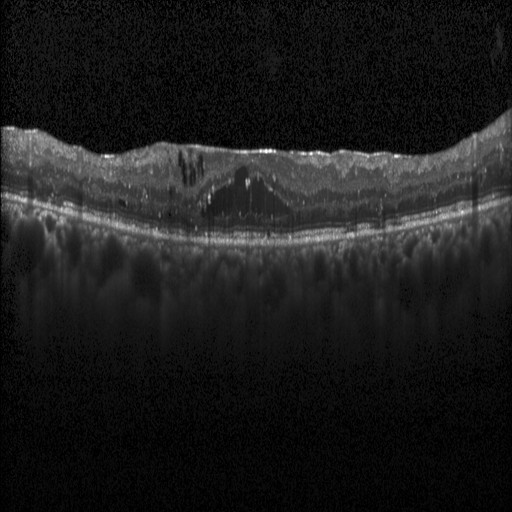 OCT B-scan.
Finding: diabetic macular edema (DME).